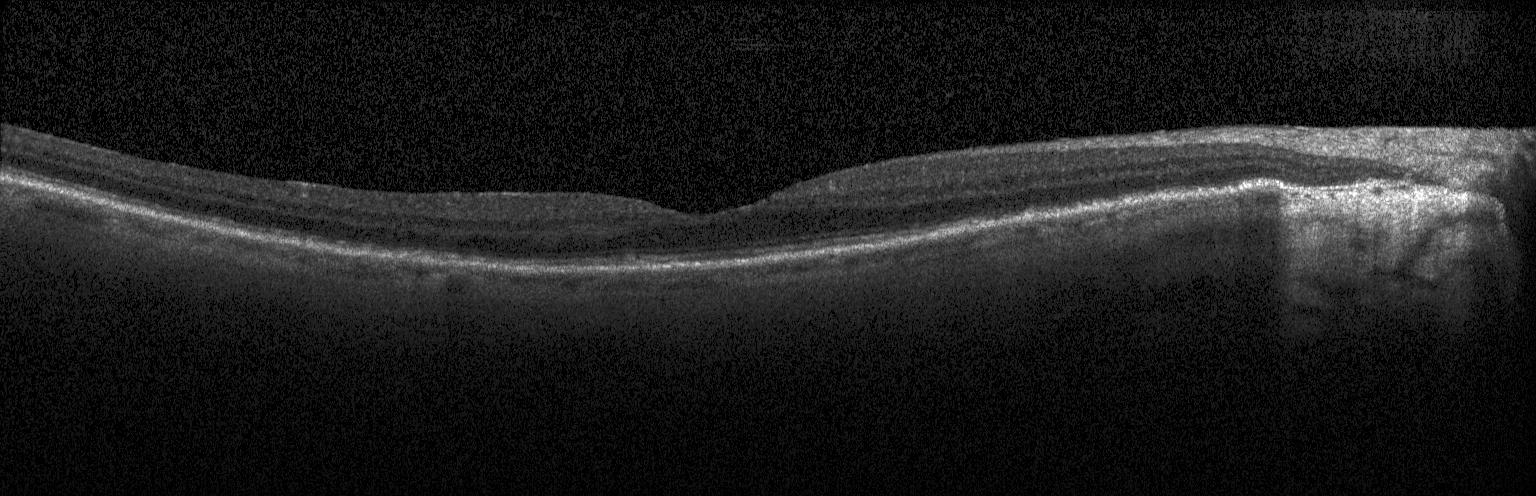 Instrument: Heidelberg Spectralis · spectral-domain OCT · retinal OCT B-scan · through the macula.
Diagnosis: no CNV, no DME, and no drusen.